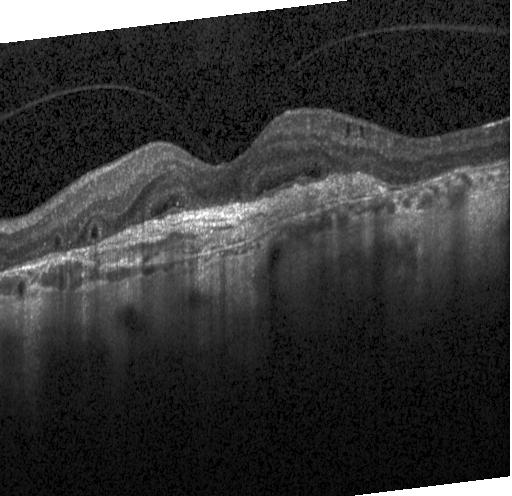
Heidelberg Spectralis; OCT B-scan; horizontal scan through the fovea.
Assessment: a choroidal neovascular membrane.